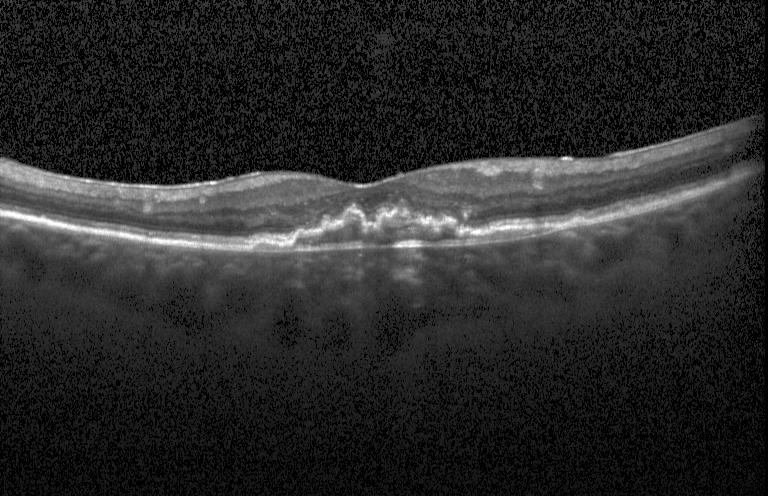
The scan shows CNV.